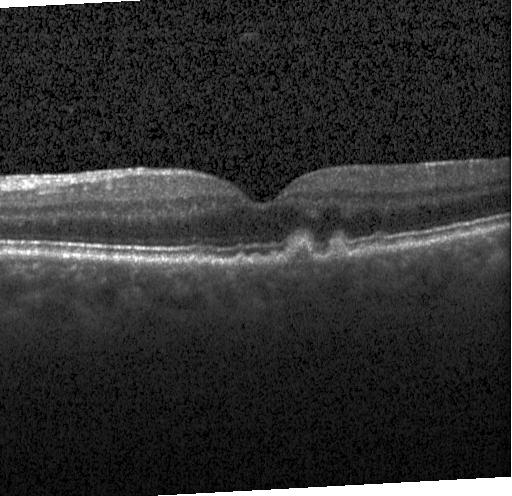
Acquired on a Heidelberg Spectralis, through the macula, spectral-domain OCT, OCT line scan. The scan shows sub-RPE drusenoid deposits.